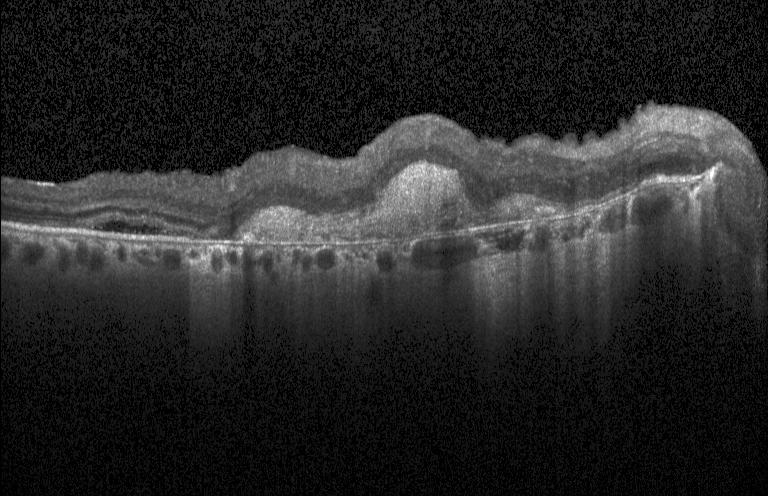

Fovea-centered, retinal OCT B-scan, SD-OCT, acquired on a Heidelberg Spectralis. A choroidal neovascular membrane.